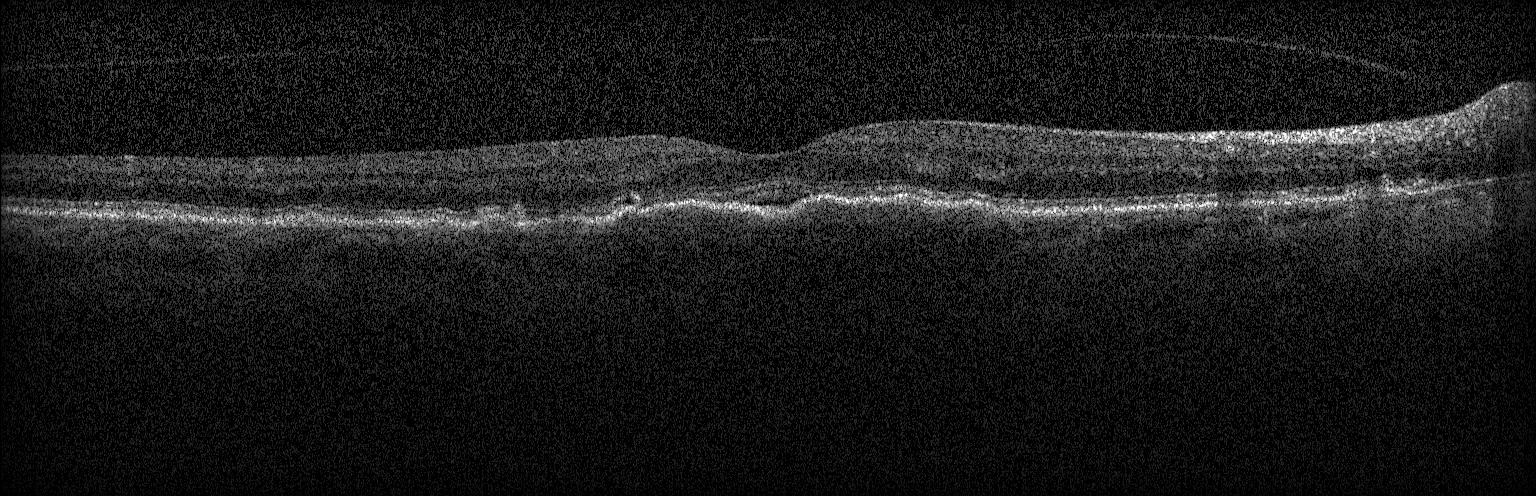

Heidelberg Spectralis · optical coherence tomography scan.
Dx: CNV.